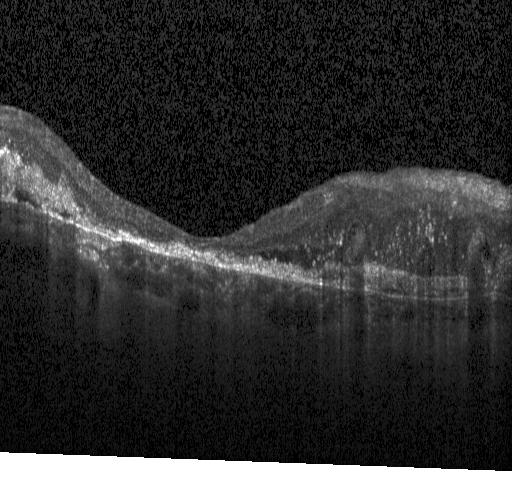 Optical coherence tomography scan. Heidelberg Spectralis — The scan shows a choroidal neovascular membrane.